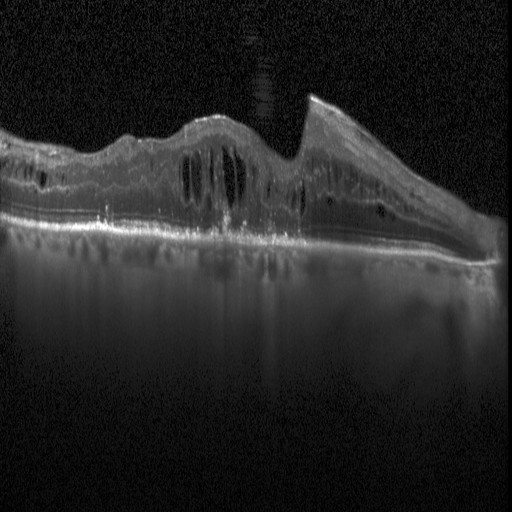
This B-scan demonstrates diabetic macular edema.